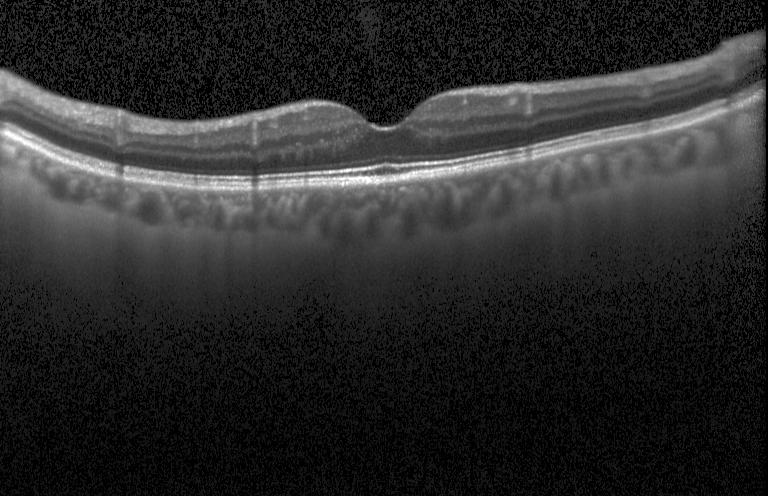 No evidence of choroidal neovascularization, diabetic macular edema, or drusen.